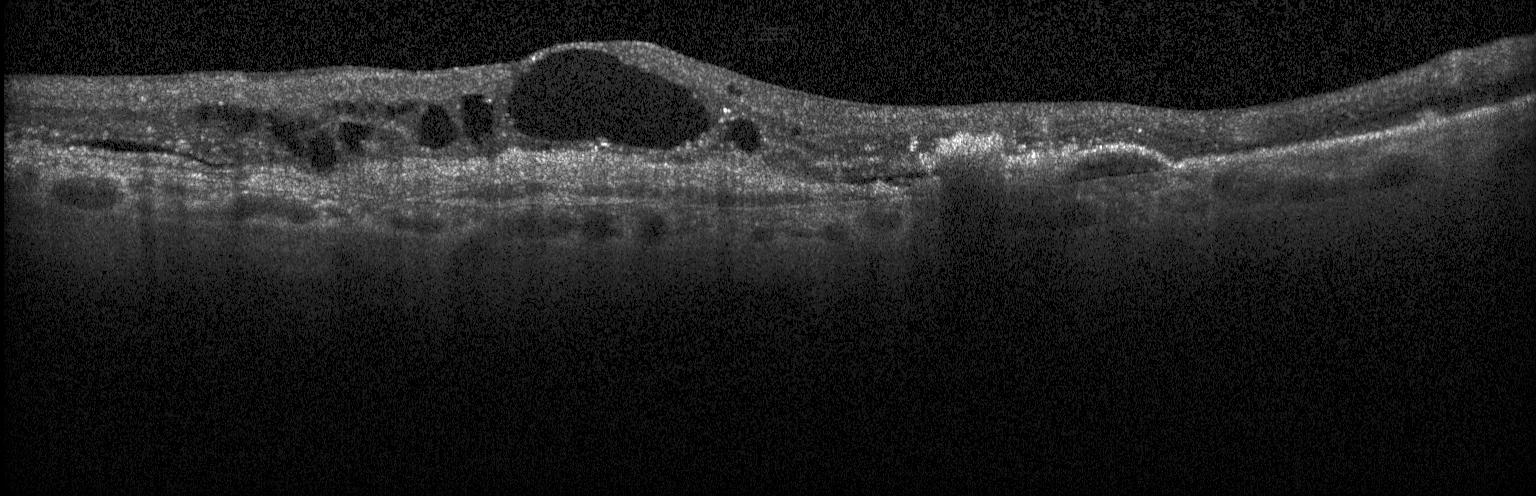 Retinal OCT B-scan · Heidelberg Spectralis OCT system · macular scan. This B-scan demonstrates a choroidal neovascular membrane.